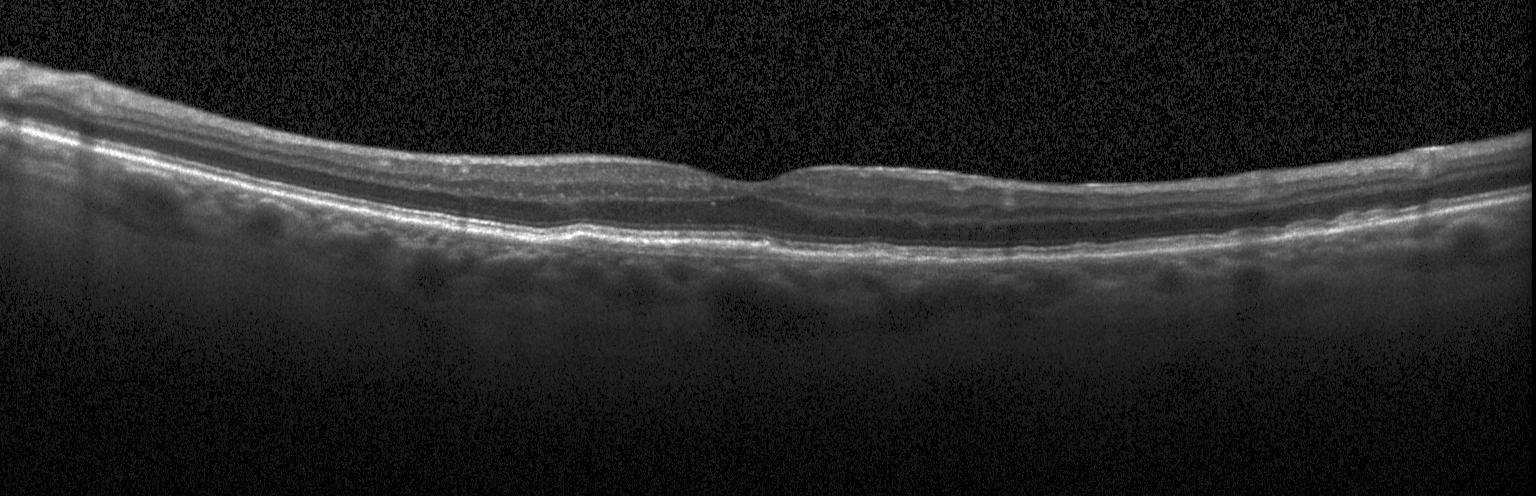
Diagnosis: choroidal neovascularization.